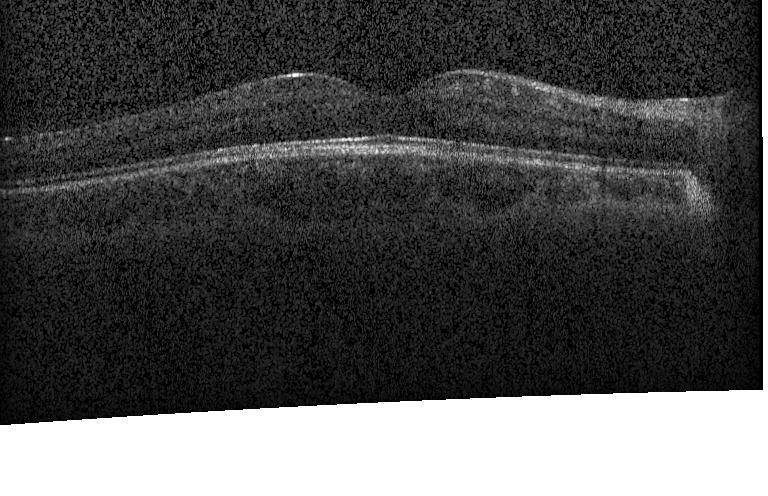

Retinal OCT B-scan.
Finding: no choroidal neovascularization, diabetic macular edema, or drusen.